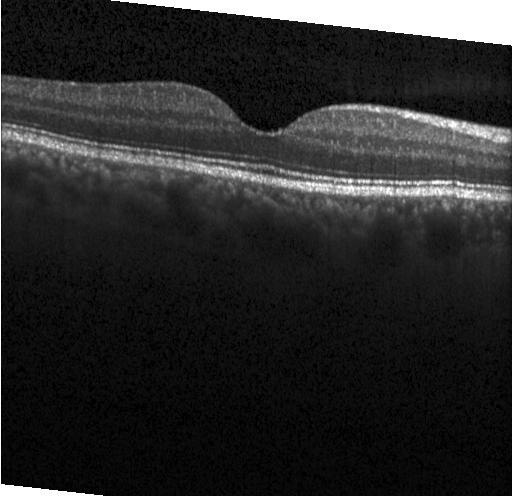

Retinal OCT cross-section · spectral-domain OCT.
Finding: no evidence of choroidal neovascularization, diabetic macular edema, or drusen.